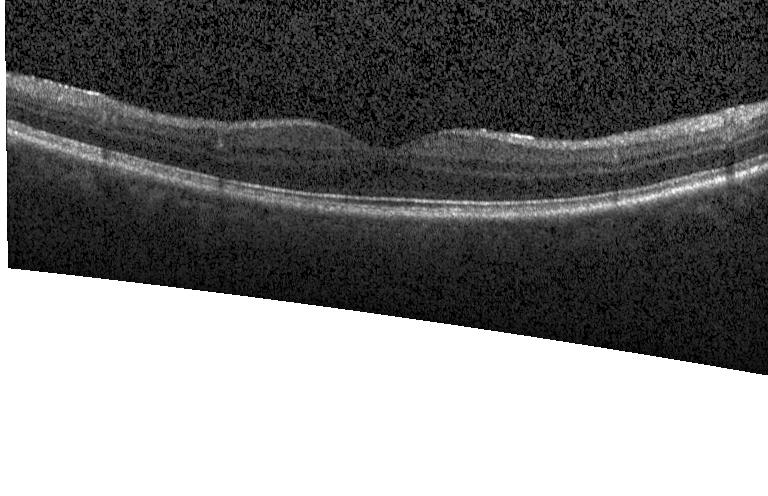

OCT B-scan
Impression: no CNV, no DME, and no drusen.